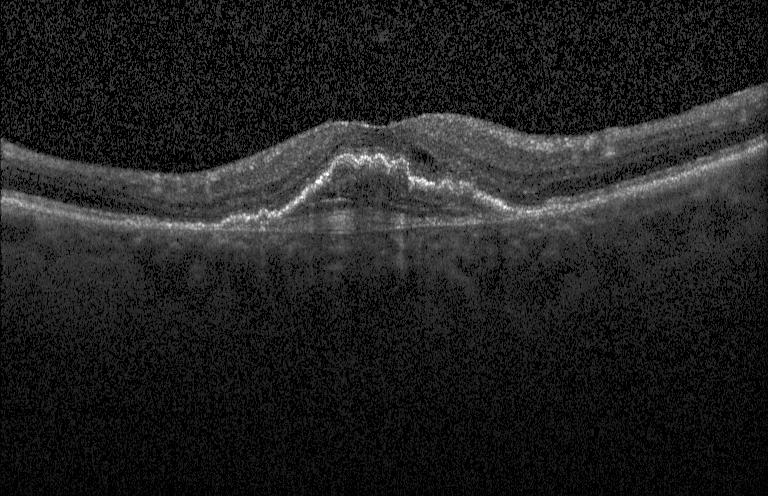
OCT line scan · macular scan · SD-OCT.
Finding: choroidal neovascularization.